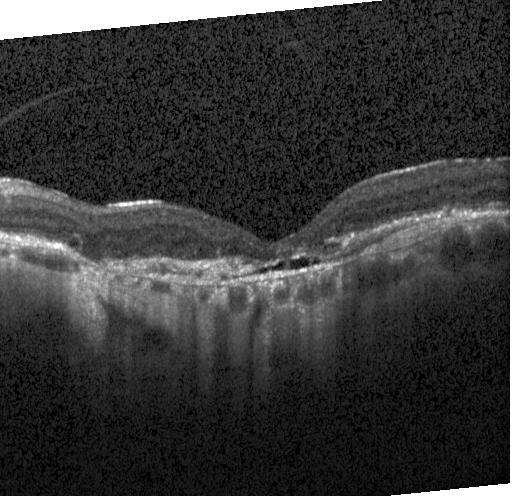 Spectral-domain OCT, retinal OCT B-scan — Impression: a choroidal neovascular membrane.